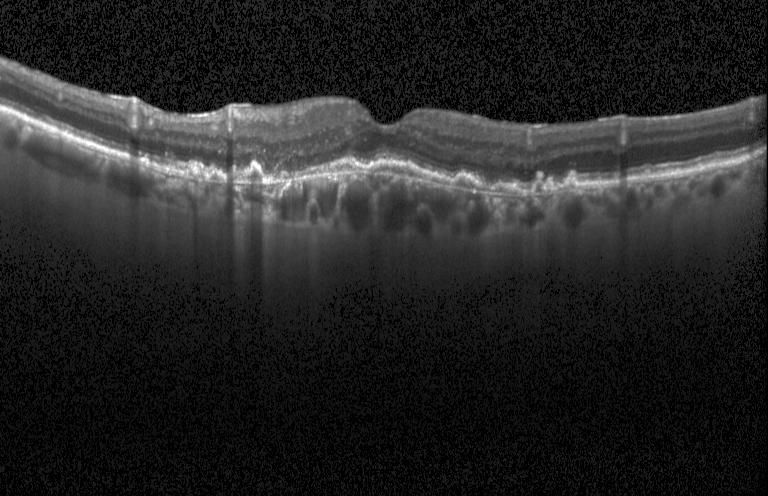

Optical coherence tomography B-scan · Heidelberg Spectralis · spectral-domain optical coherence tomography — OCT finding: a choroidal neovascular membrane.